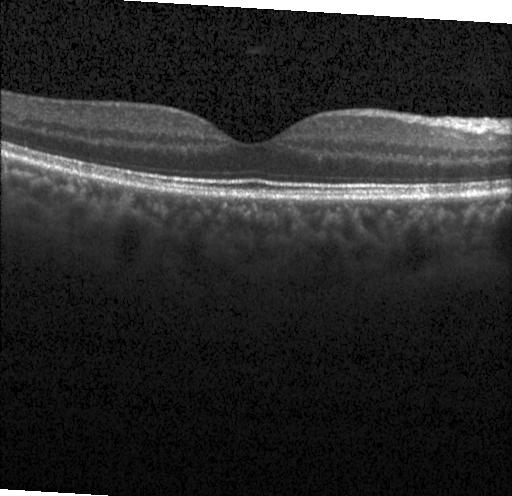 Diagnosis: no choroidal neovascularization, no diabetic macular edema, and no drusen.